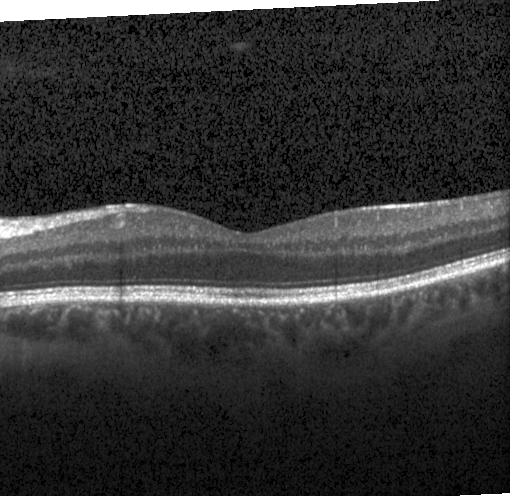
OCT scan showing neither choroidal neovascularization, diabetic macular edema, nor drusen.